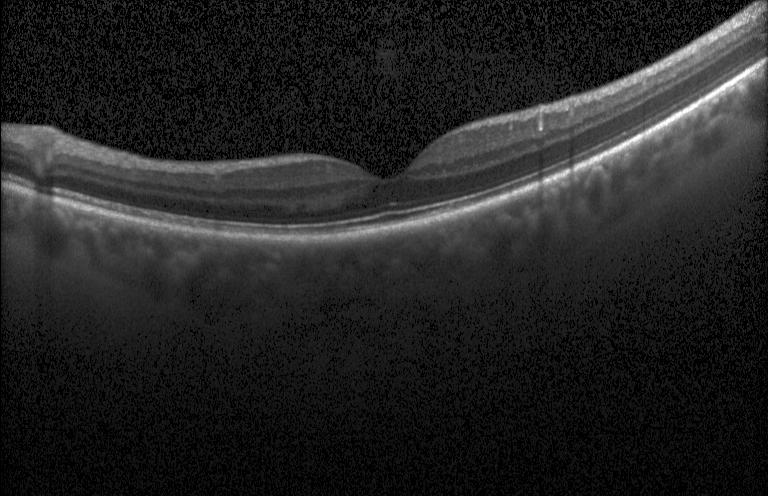

OCT scan showing no choroidal neovascularization, no diabetic macular edema, and no drusen.